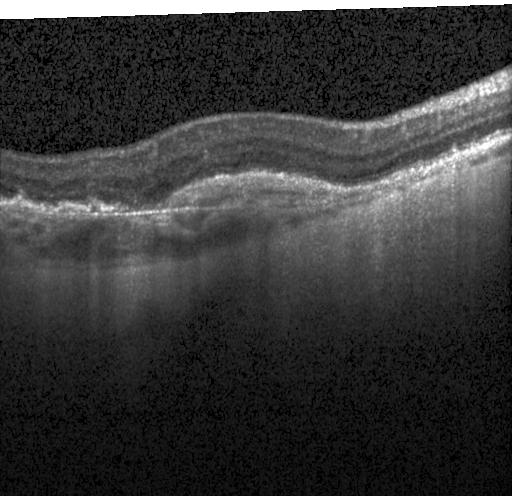

Optical coherence tomography scan · through the macula. Macular OCT: choroidal neovascularization (CNV).